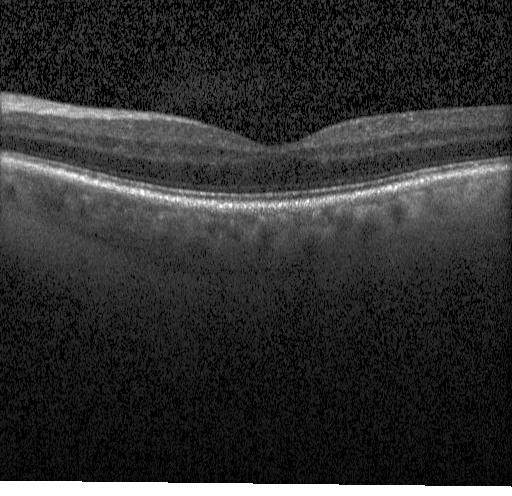

OCT line scan
Diagnosis: neither CNV, DME, nor drusen.